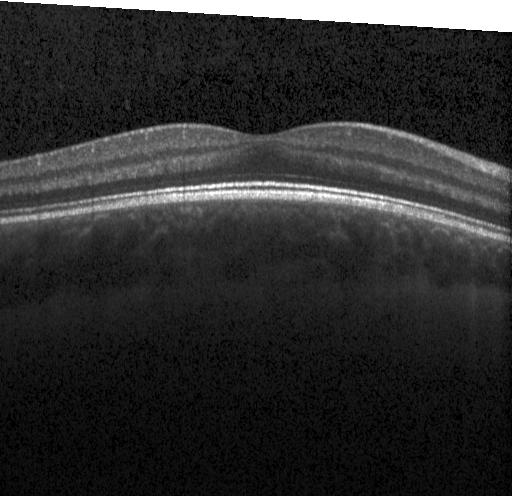 Finding: no evidence of CNV, DME, or drusen.